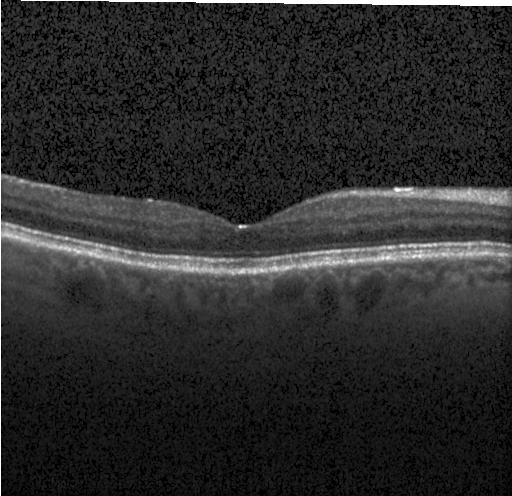
Macular OCT demonstrating no evidence of choroidal neovascularization, diabetic macular edema, or drusen.